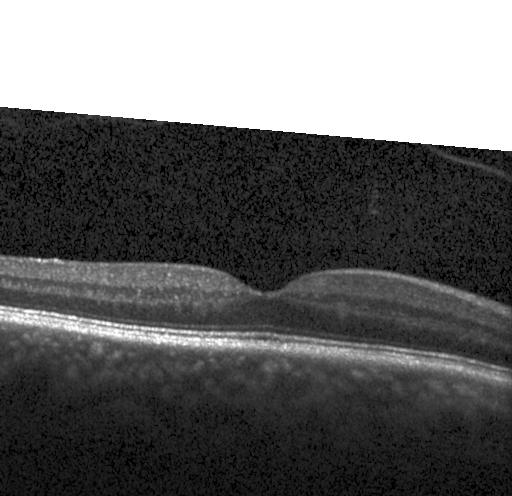
Heidelberg Spectralis. Through the macula. Retinal OCT B-scan. Dx: no choroidal neovascularization, no diabetic macular edema, and no drusen.